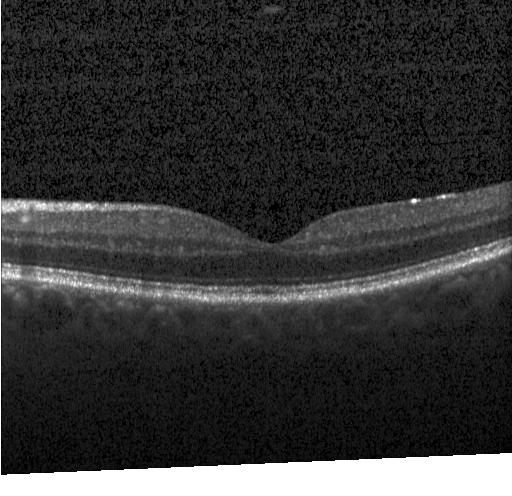 Heidelberg Spectralis OCT system, optical coherence tomography B-scan
Neither CNV, DME, nor drusen.